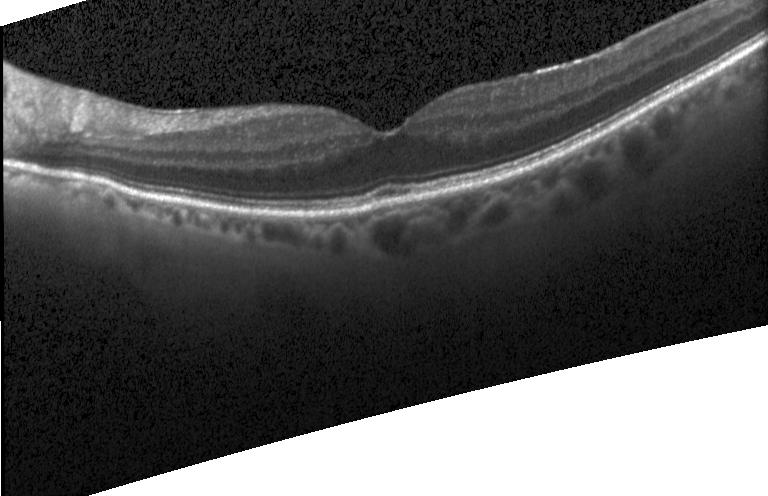
Optical coherence tomography scan; fovea-centered; acquired on a Heidelberg Spectralis; spectral-domain optical coherence tomography — Diagnosis: neither CNV, DME, nor drusen.